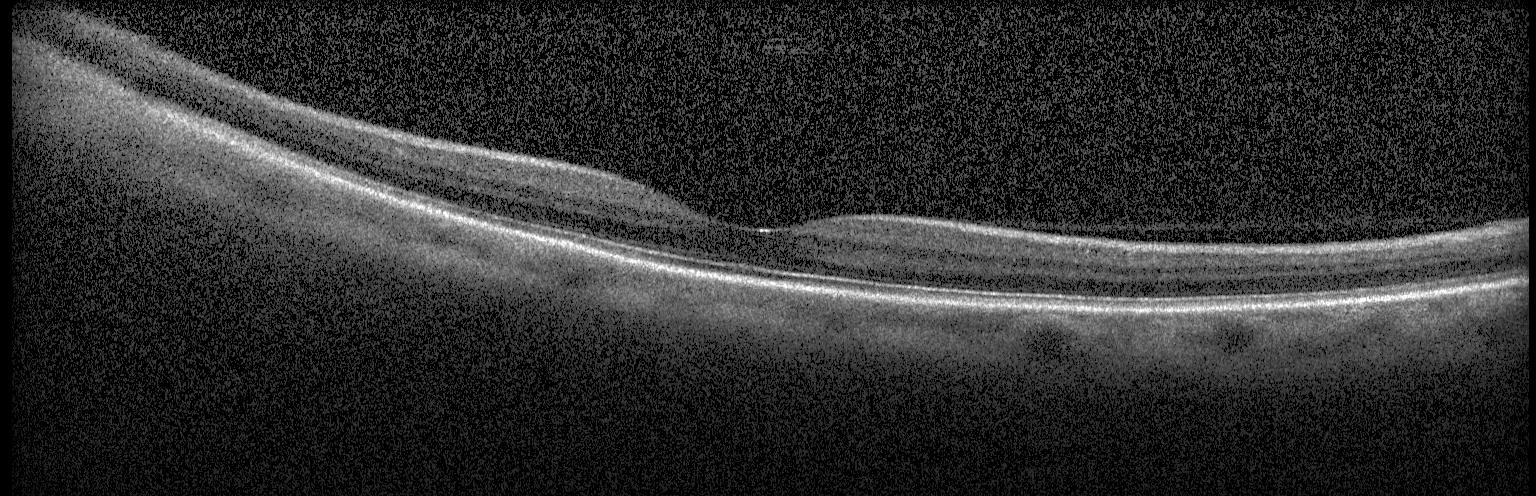

Finding: no evidence of choroidal neovascularization, diabetic macular edema, or drusen.